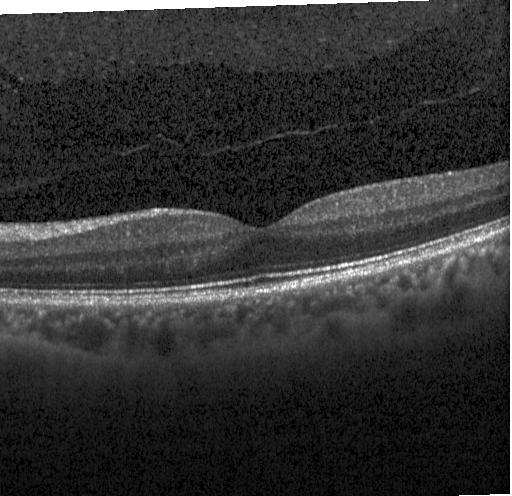

OCT line scan · fovea-centered · spectral-domain OCT · Heidelberg Spectralis — Diagnosis: neither choroidal neovascularization, diabetic macular edema, nor drusen.